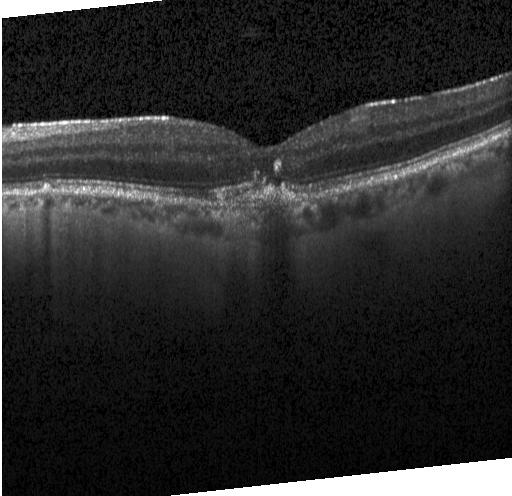
OCT B-scan; horizontal scan through the fovea; instrument: Heidelberg Spectralis; SD-OCT.
Impression: a choroidal neovascular membrane.